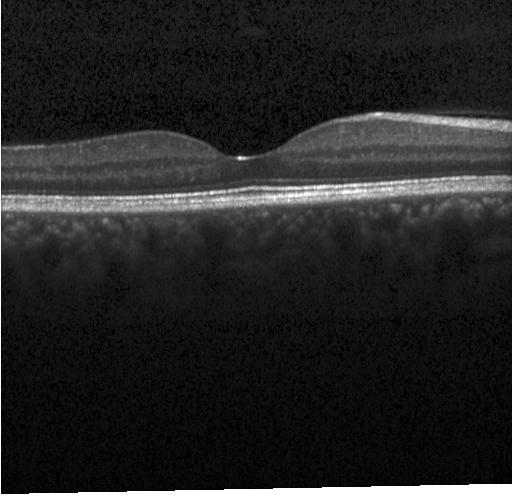

OCT B-scan.
Dx: no choroidal neovascularization, diabetic macular edema, or drusen.